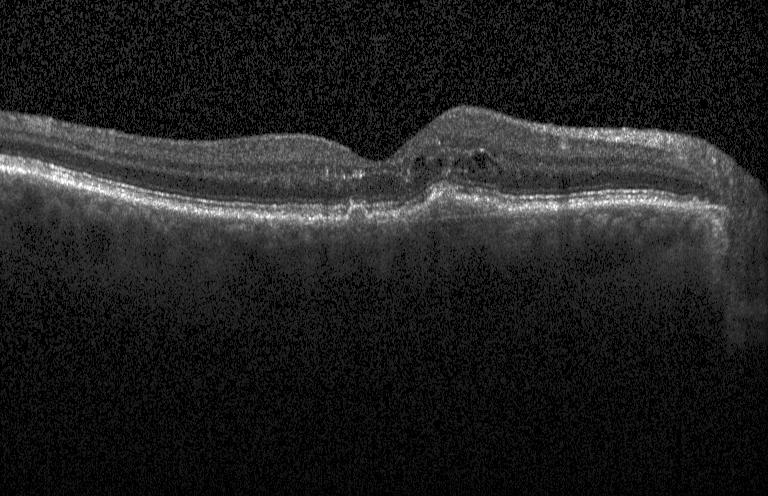

SD-OCT, through the macula, Heidelberg Spectralis OCT system, OCT B-scan — OCT finding: choroidal neovascularization.